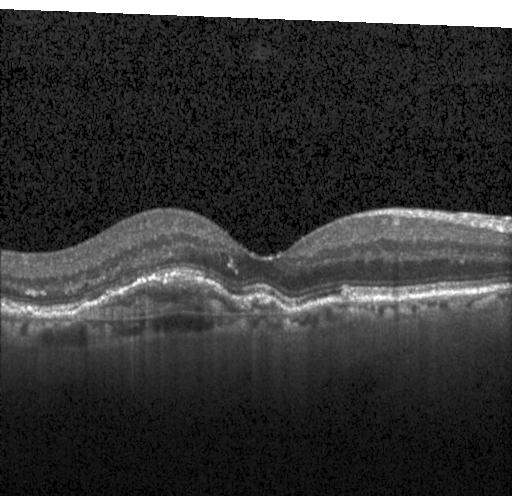

Retinal OCT cross-section showing a choroidal neovascular membrane.